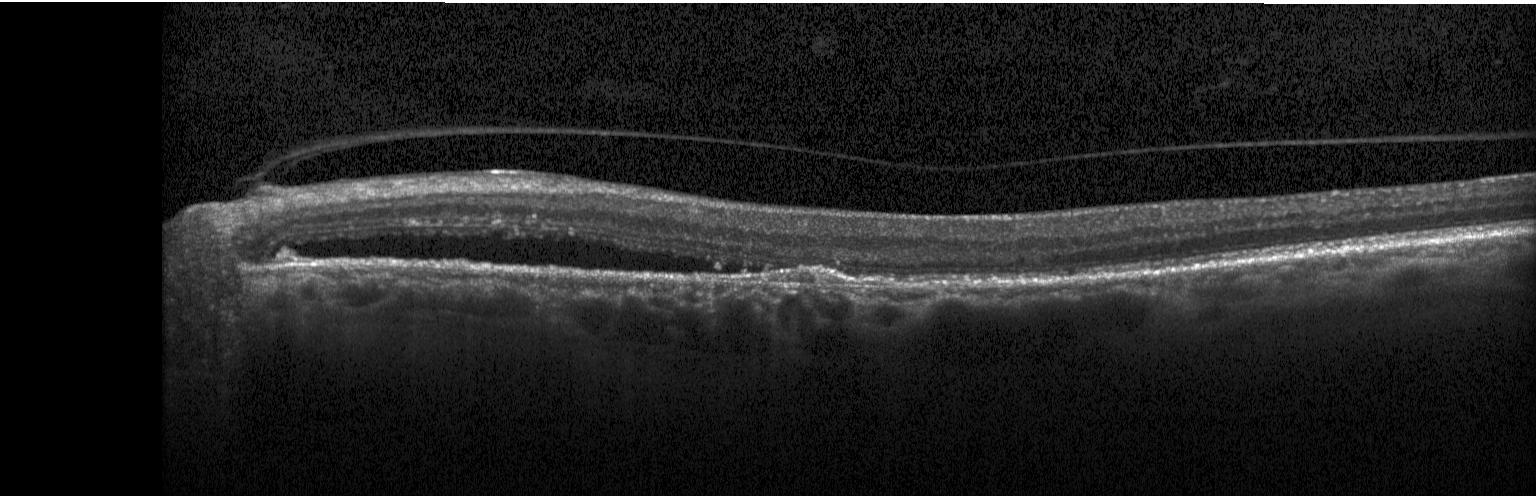

Optical coherence tomography scan.
The scan shows CNV.